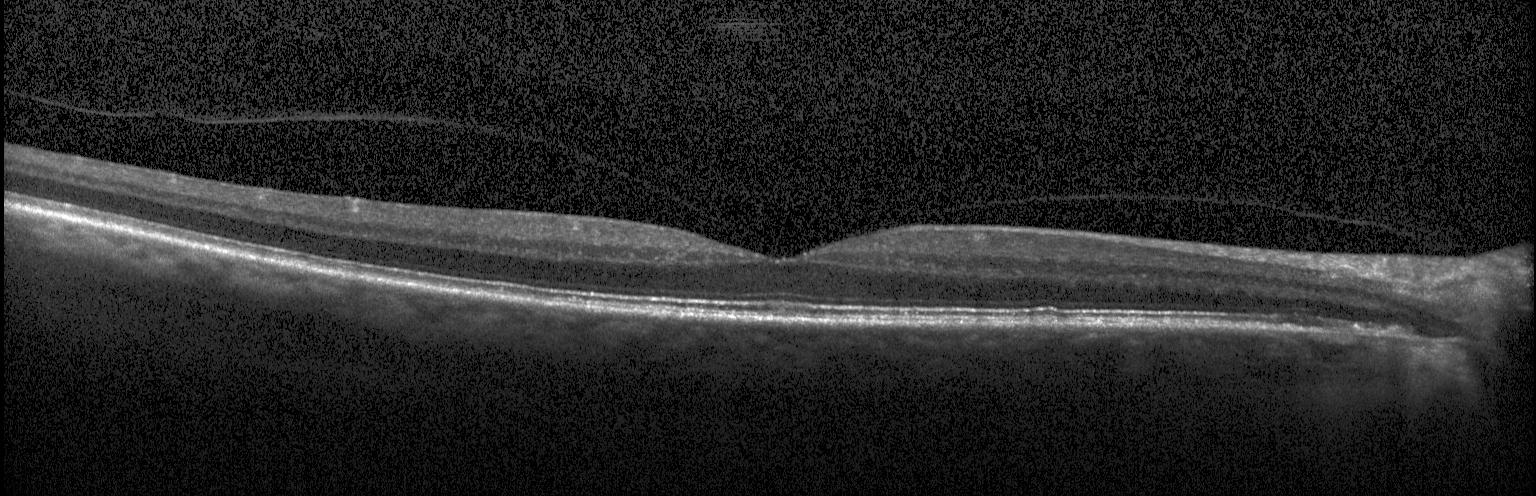

Heidelberg Spectralis · optical coherence tomography B-scan. Assessment: no CNV, DME, or drusen.